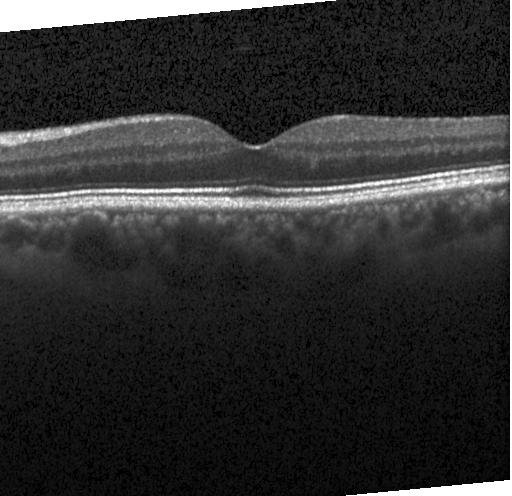
OCT B-scan.
This B-scan demonstrates no choroidal neovascularization, diabetic macular edema, or drusen.